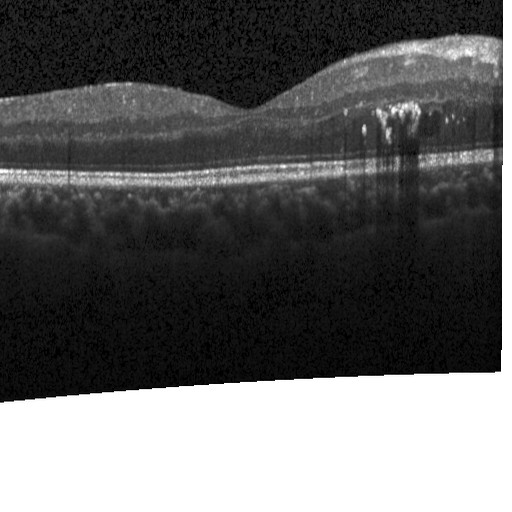 Optical coherence tomography B-scan. Finding: diabetic macular edema.